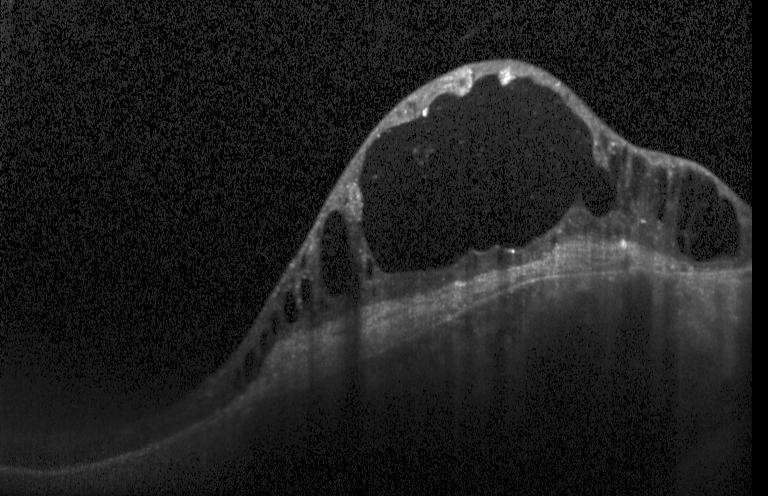 Diagnosis: a choroidal neovascular membrane.